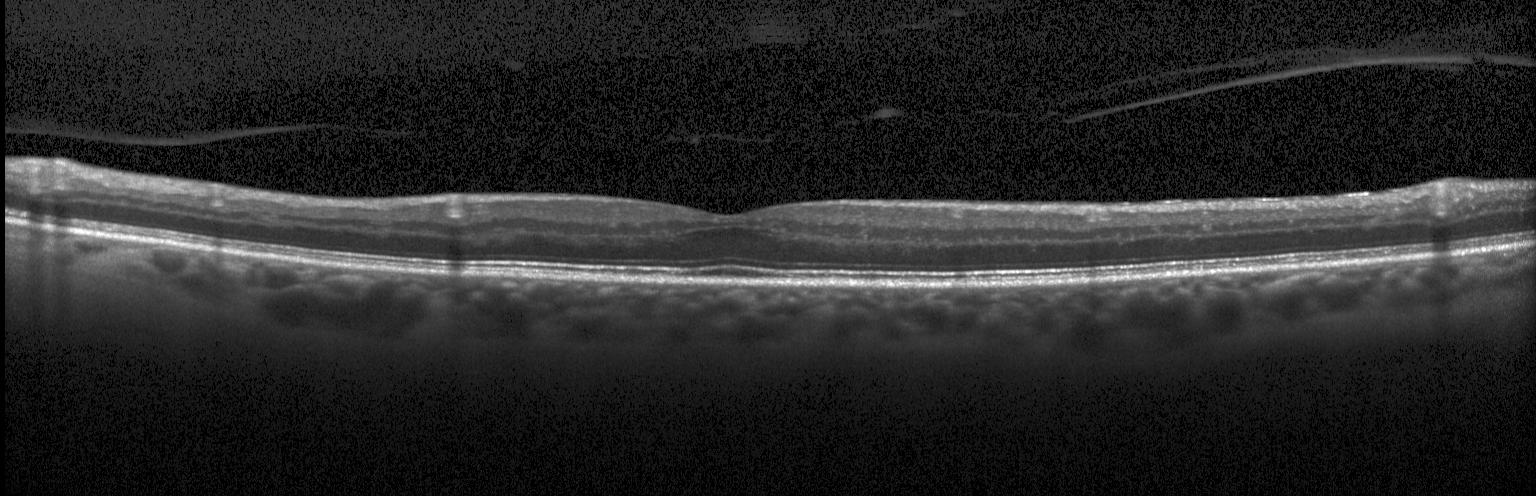
OCT B-scan
Diagnosis: no evidence of choroidal neovascularization, diabetic macular edema, or drusen.